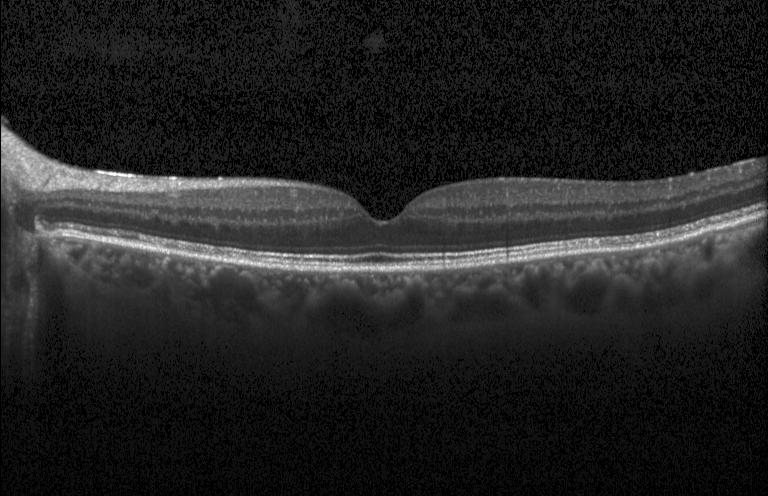 Optical coherence tomography scan.
Finding: no choroidal neovascularization, diabetic macular edema, or drusen.